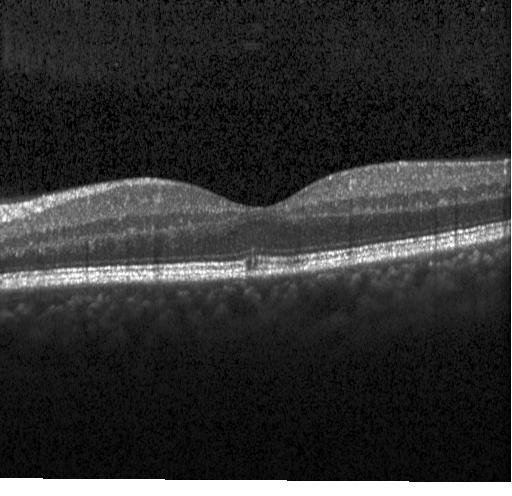
Optical coherence tomography scan · fovea-centered · Heidelberg Spectralis.
Impression: no evidence of CNV, DME, or drusen.